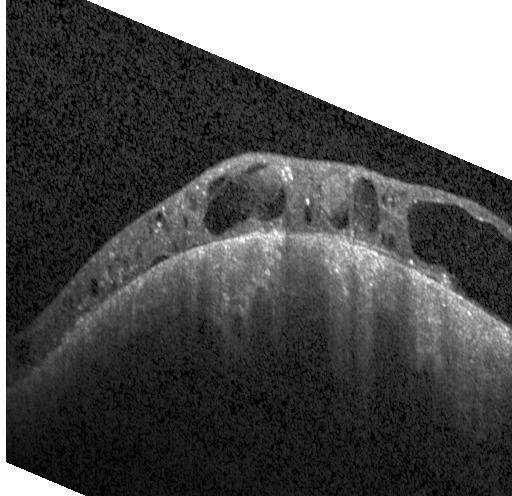 Spectral-domain OCT B-scan: diabetic macular edema.